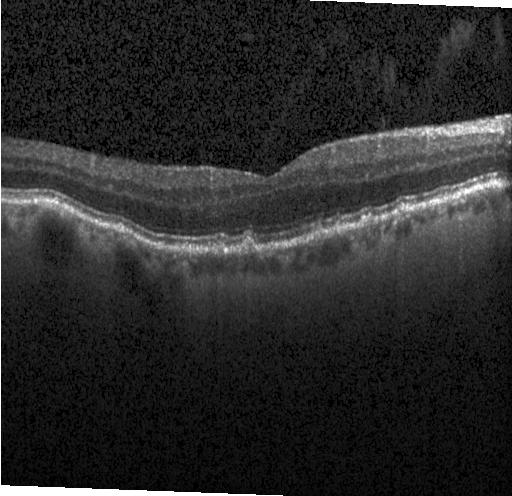

Retinal OCT cross-section showing sub-RPE drusenoid deposits.